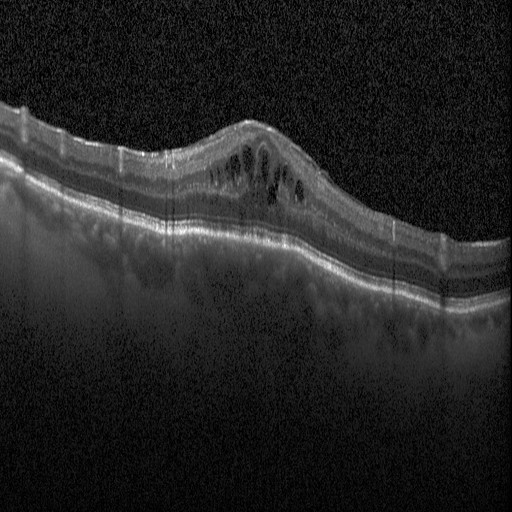

Instrument: Heidelberg Spectralis · optical coherence tomography scan · macular scan · spectral-domain OCT. The scan shows diabetic macular edema.